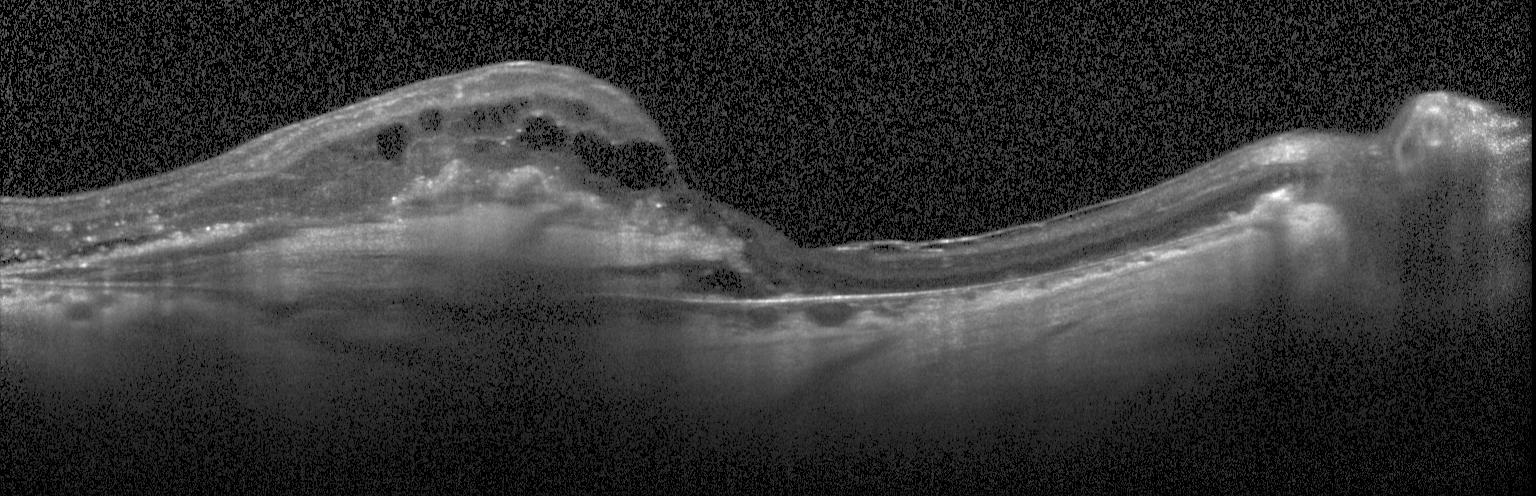 OCT B-scan · macular scan · spectral-domain optical coherence tomography.
Dx: CNV.